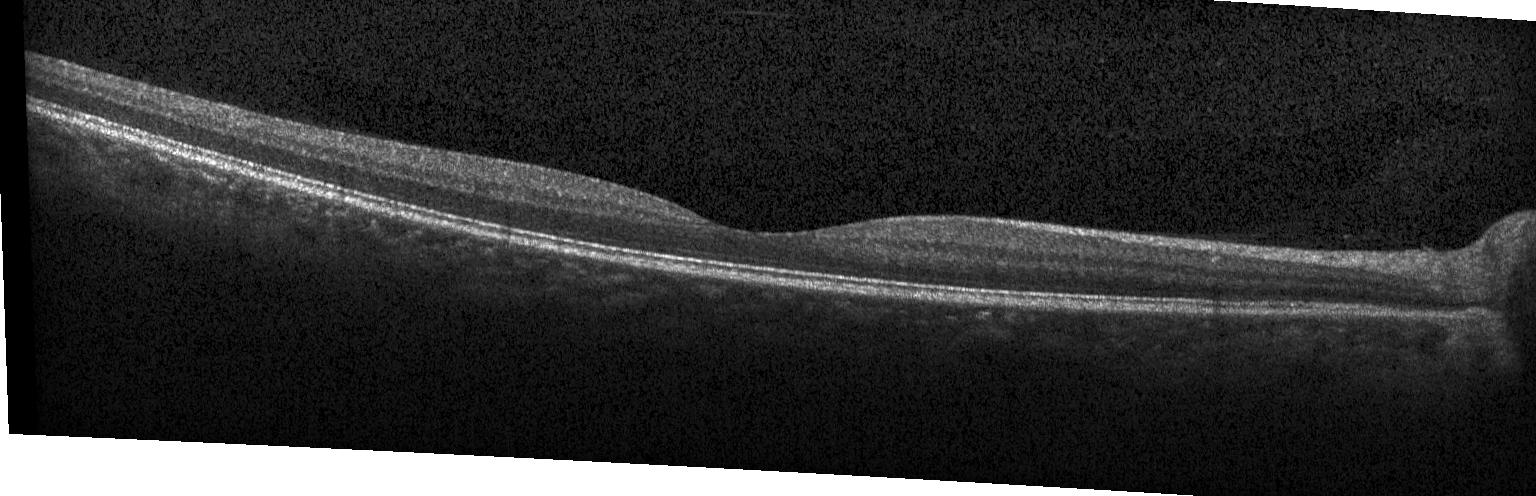 Instrument: Heidelberg Spectralis; spectral-domain optical coherence tomography; retinal OCT cross-section
Impression: no choroidal neovascularization, no diabetic macular edema, and no drusen.